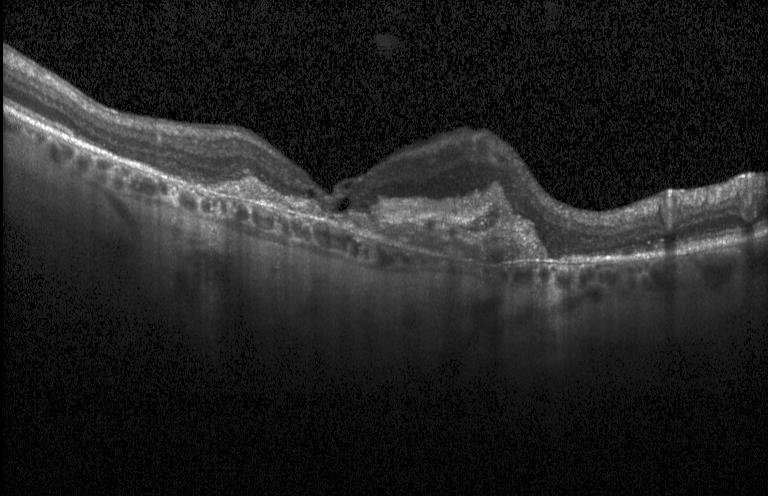

Through the macula. Spectral-domain OCT. OCT B-scan — A choroidal neovascular membrane.